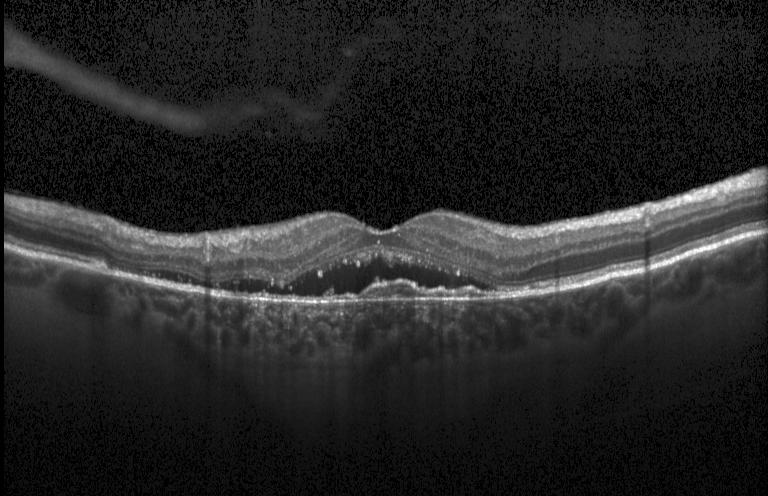 Retinal OCT cross-section showing choroidal neovascularization.